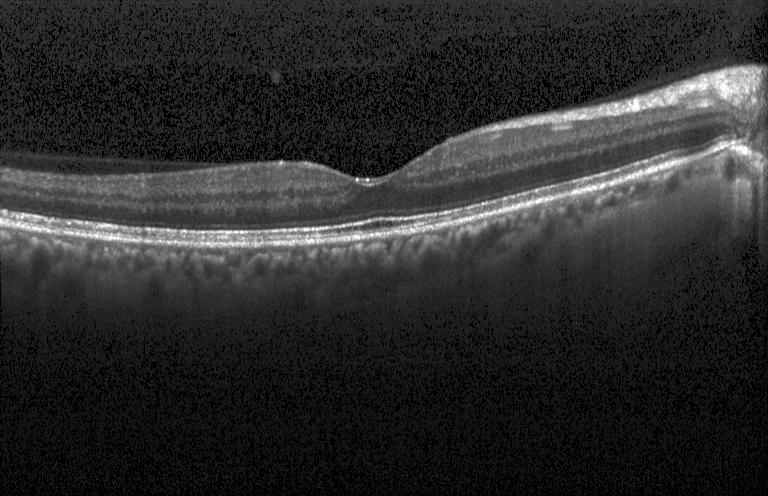
Spectral-domain optical coherence tomography · centered on the fovea · acquired on a Heidelberg Spectralis · OCT B-scan.
Diagnosis: neither CNV, DME, nor drusen.